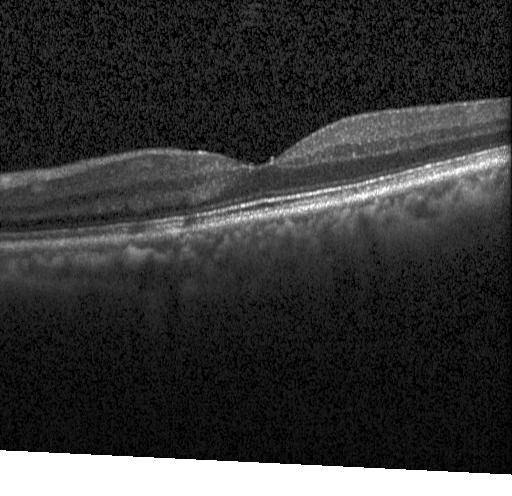

OCT finding: no CNV, no DME, and no drusen.